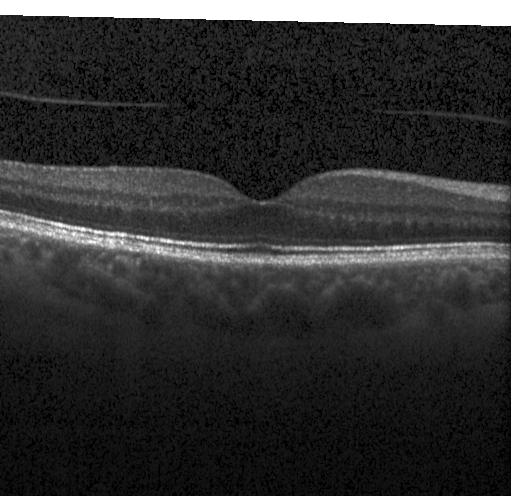
Dx: no choroidal neovascularization, no diabetic macular edema, and no drusen.